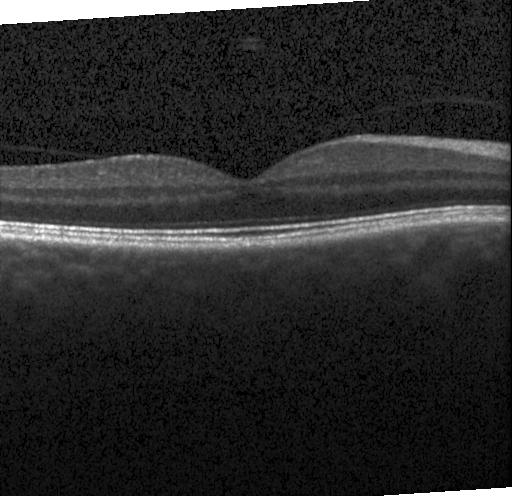

Retinal OCT cross-section — Dx: no choroidal neovascularization, diabetic macular edema, or drusen.